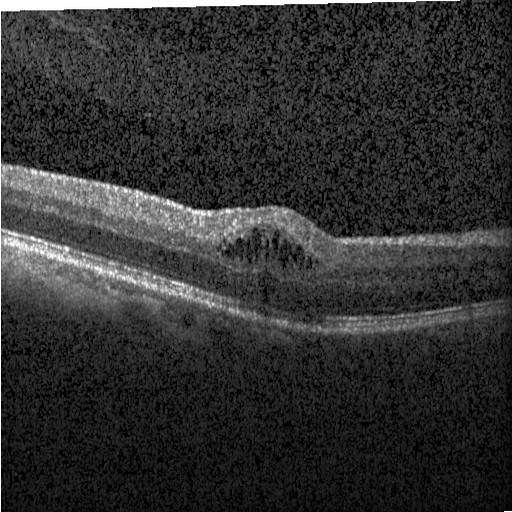

Optical coherence tomography scan — The scan shows DME.